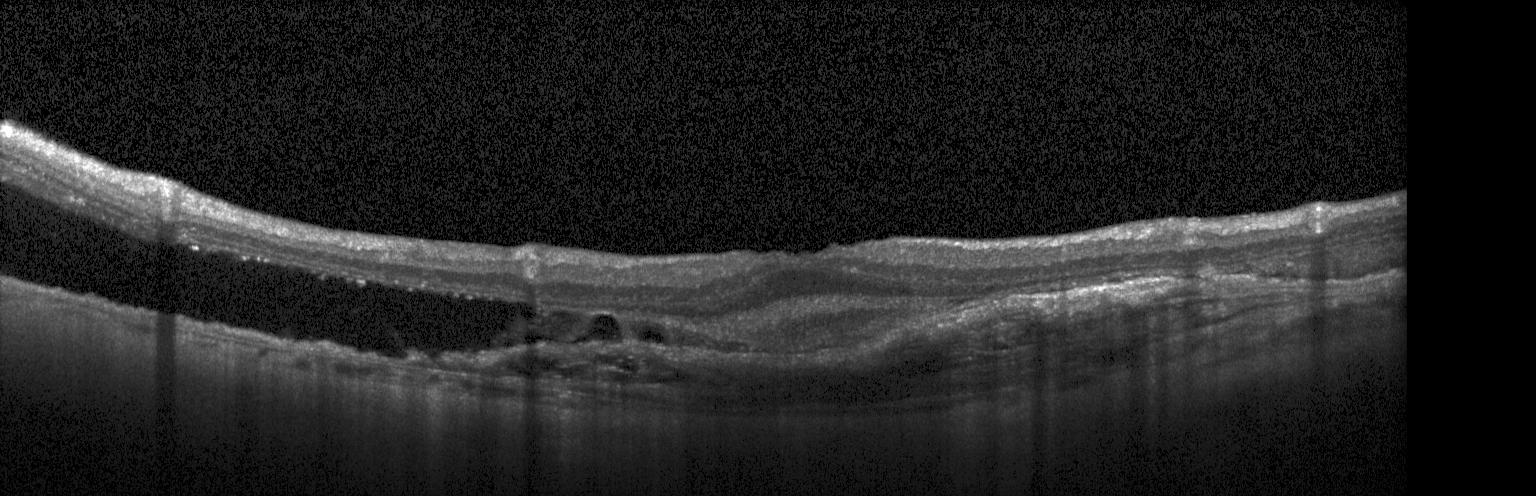

Macular OCT demonstrating a choroidal neovascular membrane.